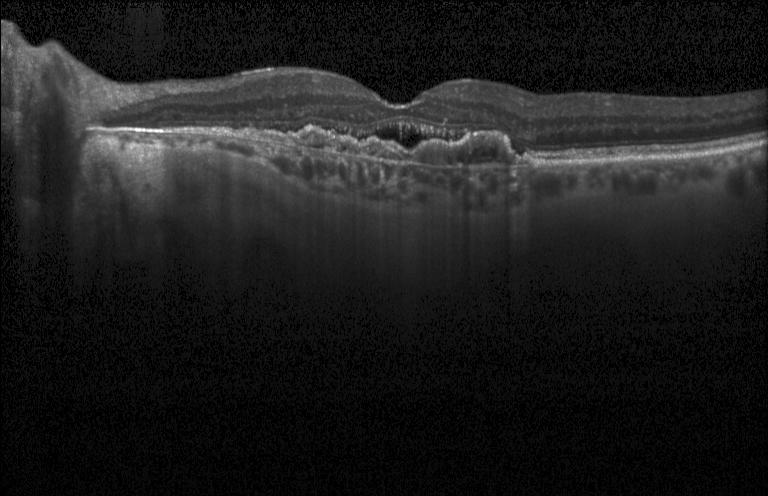

Optical coherence tomography B-scan. This B-scan demonstrates CNV.